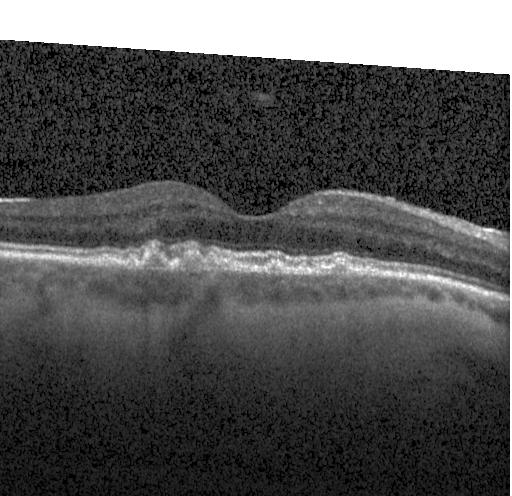 Optical coherence tomography scan. Heidelberg Spectralis. Finding: drusen.